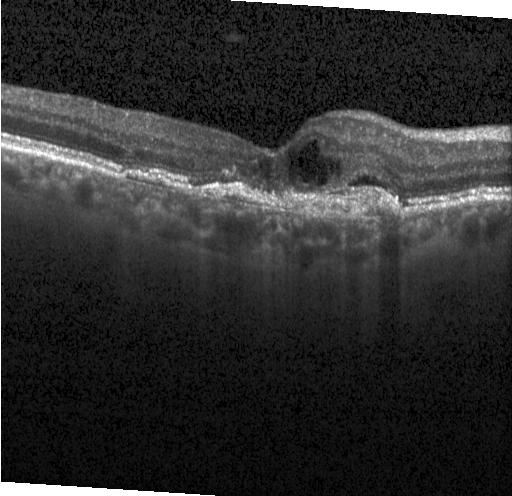 Acquired on a Heidelberg Spectralis · through the macula · retinal OCT cross-section. Diagnosis: a choroidal neovascular membrane.